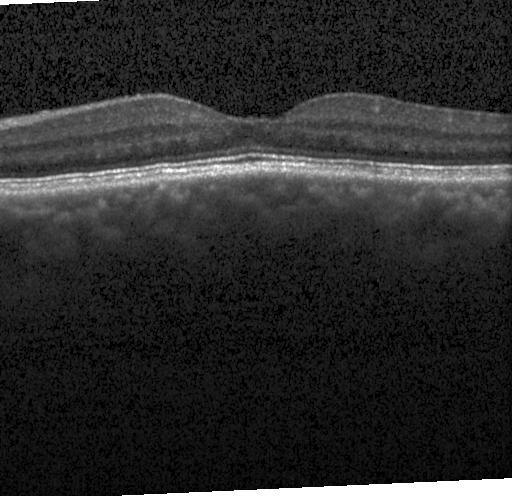 Optical coherence tomography scan, fovea-centered, instrument: Heidelberg Spectralis, spectral-domain OCT — Dx: no choroidal neovascularization, no diabetic macular edema, and no drusen.